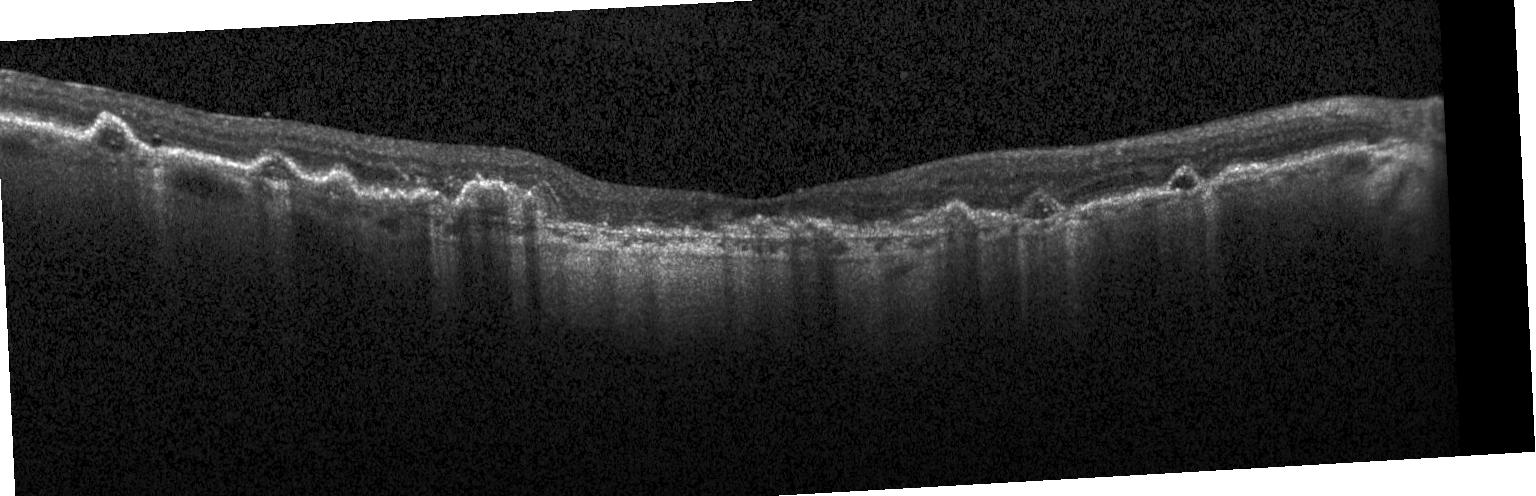
OCT line scan.
Finding: a choroidal neovascular membrane.